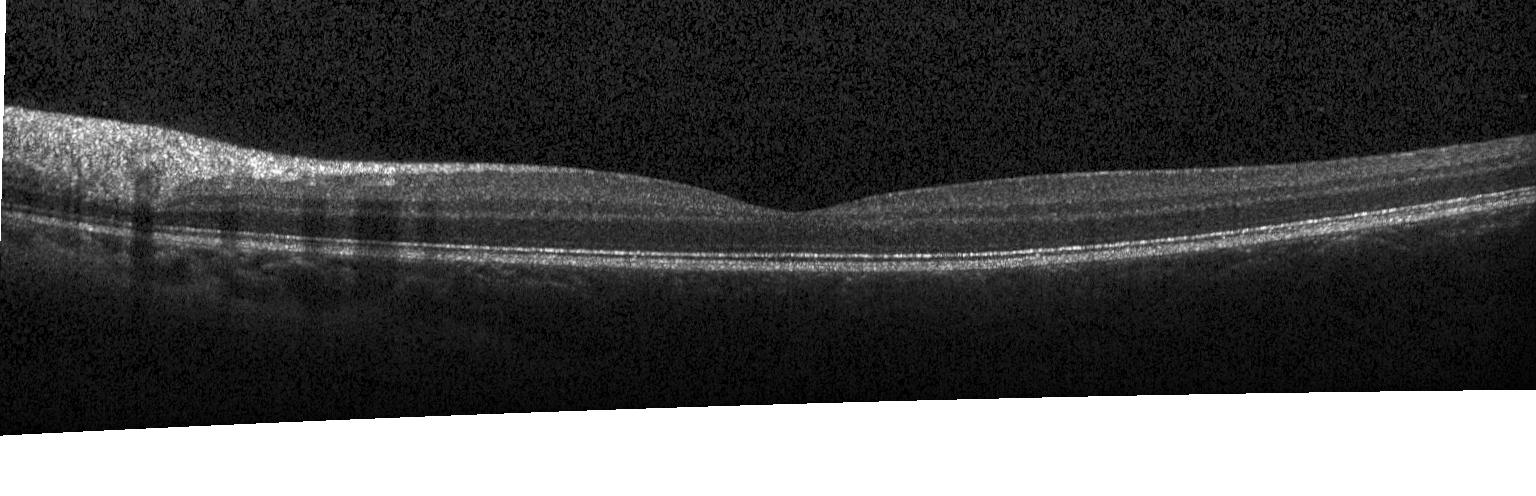

Acquired on a Heidelberg Spectralis. OCT line scan. Centered on the fovea — Assessment: neither CNV, DME, nor drusen.